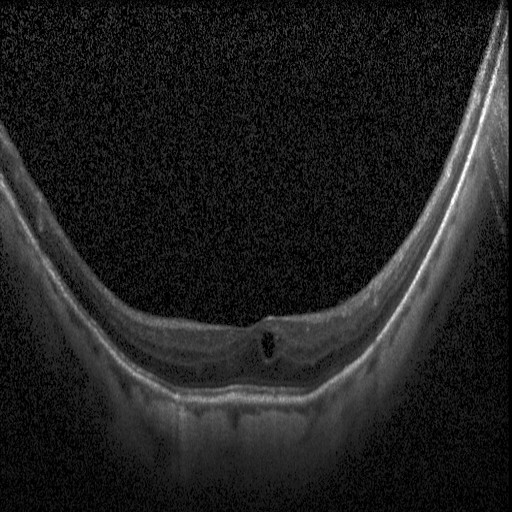 Finding: diabetic macular edema (DME).